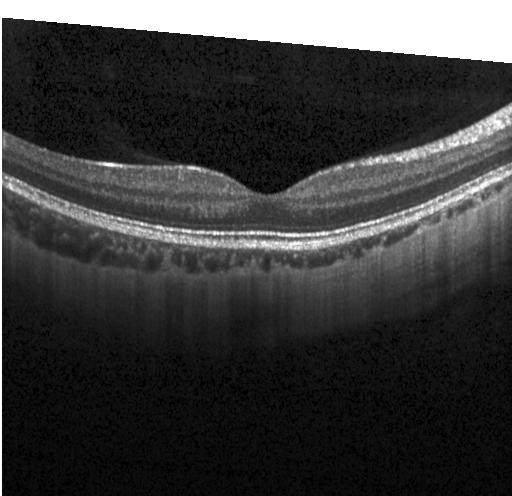
Diagnosis: no evidence of choroidal neovascularization, diabetic macular edema, or drusen.